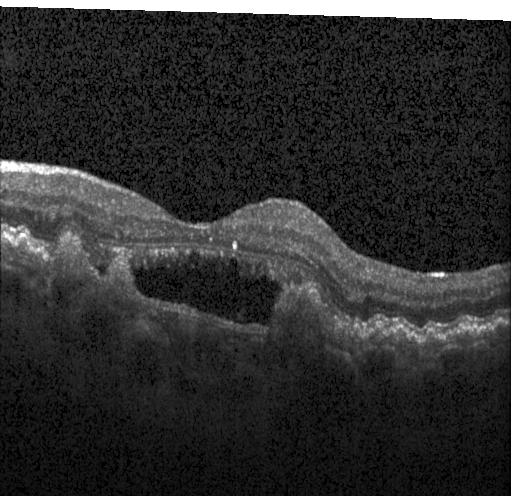

Diagnosis: a choroidal neovascular membrane.